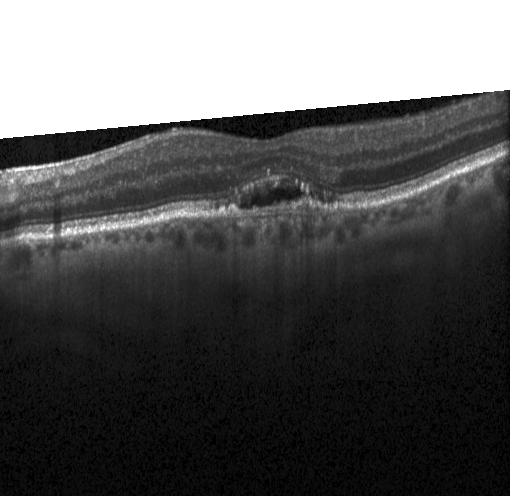
Finding: a choroidal neovascular membrane.